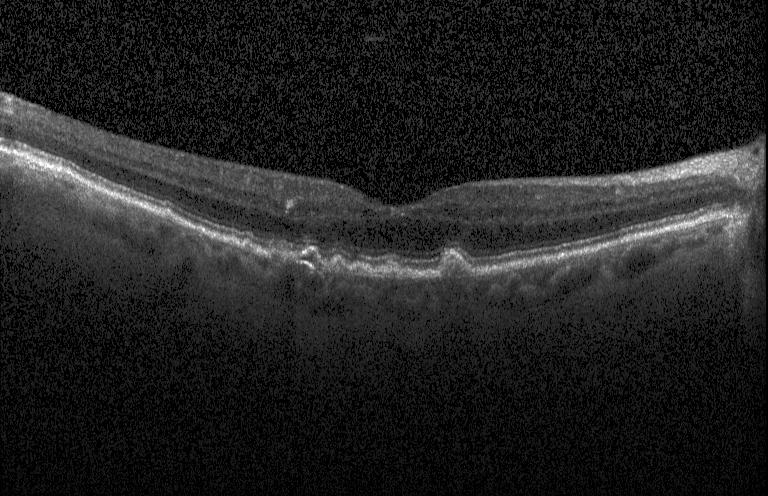 Optical coherence tomography B-scan, fovea-centered
Finding: drusen.